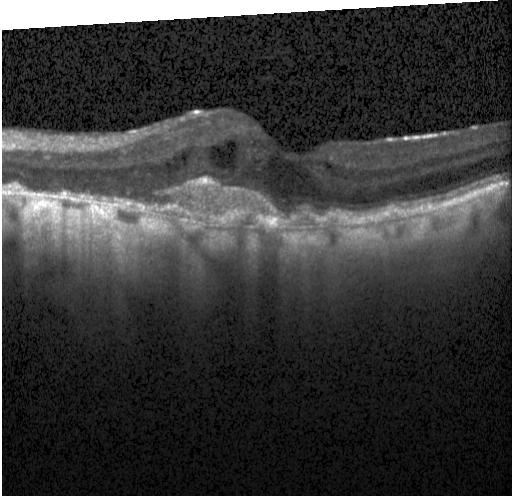

Optical coherence tomography B-scan
A choroidal neovascular membrane.